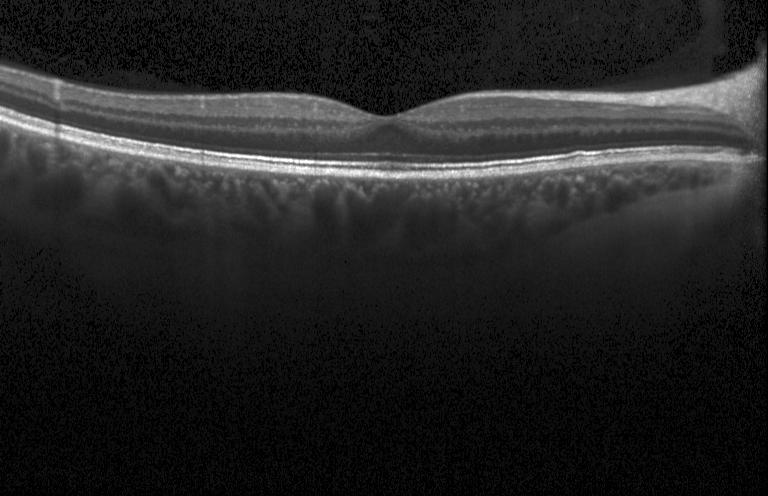 Spectral-domain OCT · Heidelberg Spectralis OCT system · OCT line scan · through the macula
Finding: neither CNV, DME, nor drusen.